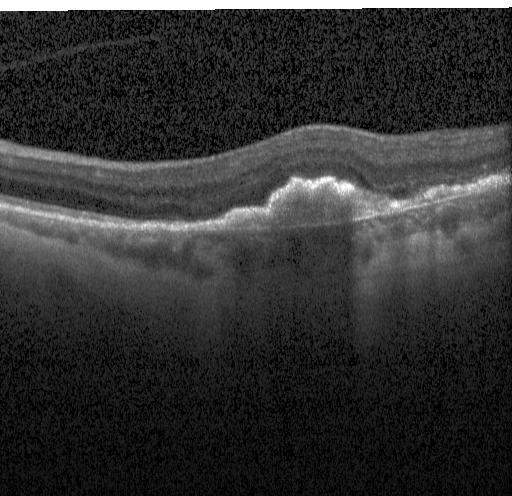 This B-scan demonstrates choroidal neovascularization (CNV).